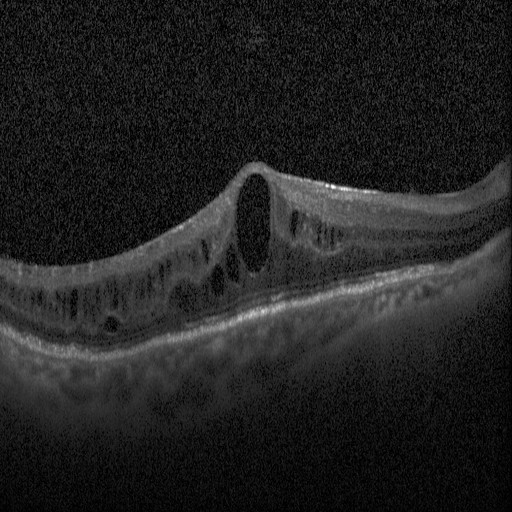
Optical coherence tomography scan. Fovea-centered. Acquired on a Heidelberg Spectralis — Diagnosis: diabetic macular edema (DME).